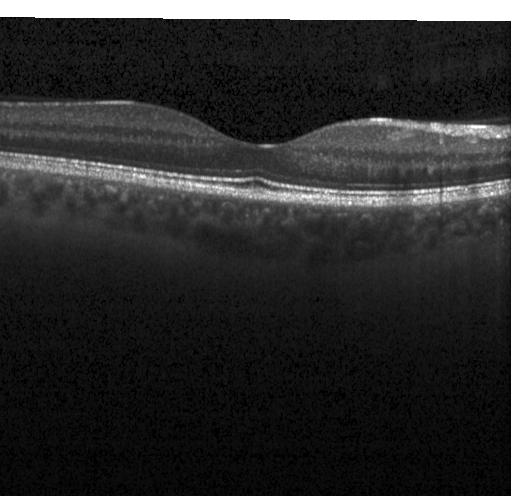
Macular scan, optical coherence tomography B-scan, spectral-domain OCT — OCT finding: no CNV, DME, or drusen.